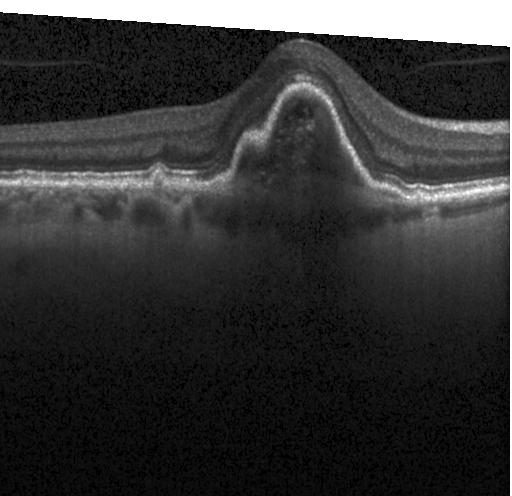 Retinal OCT cross-section. Finding: choroidal neovascularization.